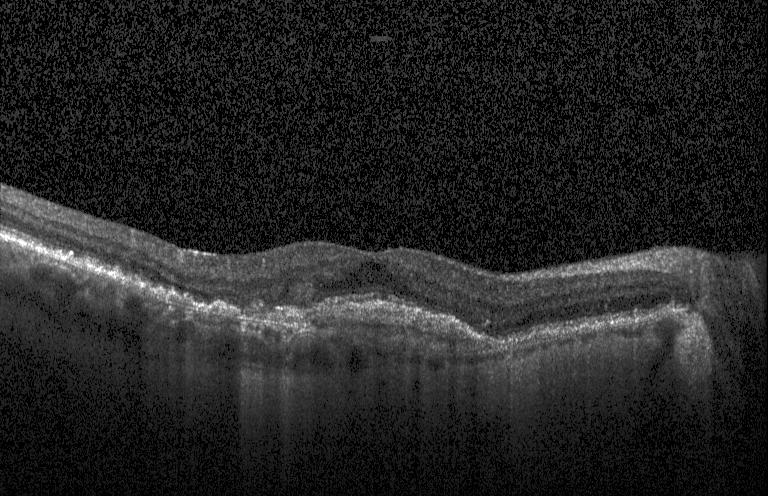 Dx: a choroidal neovascular membrane.